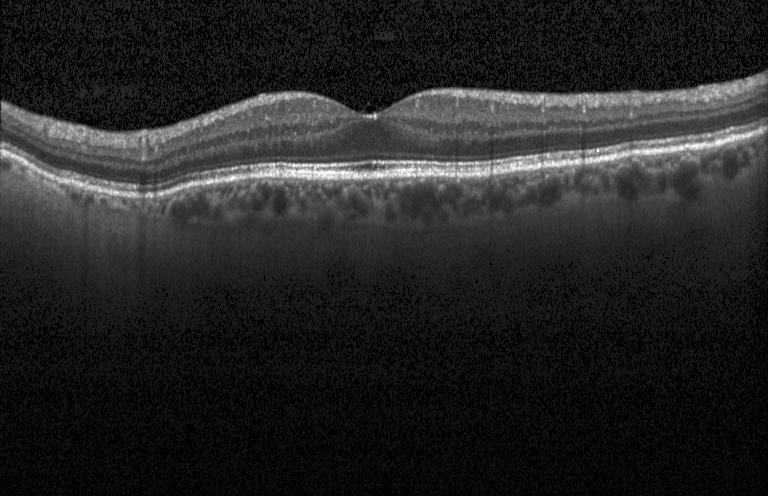

This B-scan demonstrates no evidence of choroidal neovascularization, diabetic macular edema, or drusen.